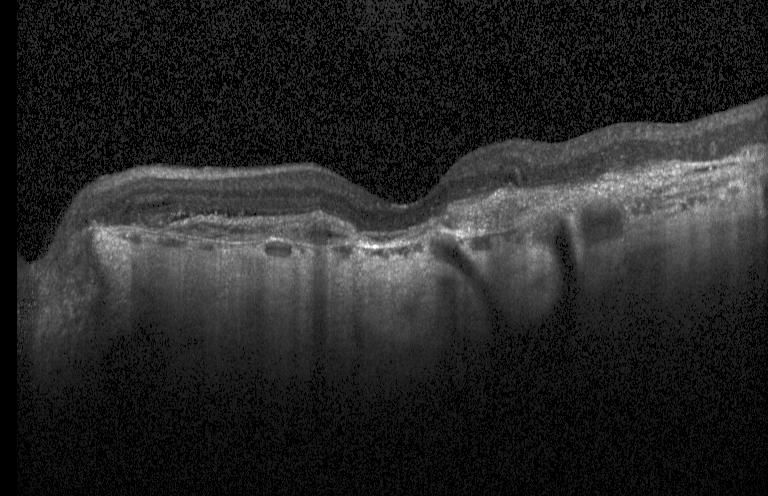
Heidelberg Spectralis OCT system; horizontal scan through the fovea; optical coherence tomography B-scan; SD-OCT.
A choroidal neovascular membrane.